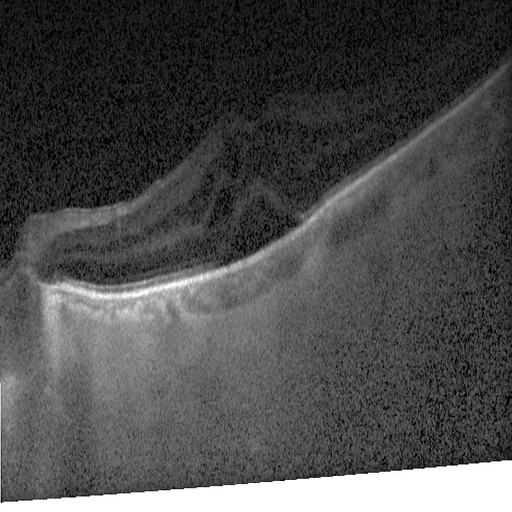
OCT line scan · Heidelberg Spectralis OCT system · centered on the fovea · SD-OCT
Diagnosis: diabetic macular edema.